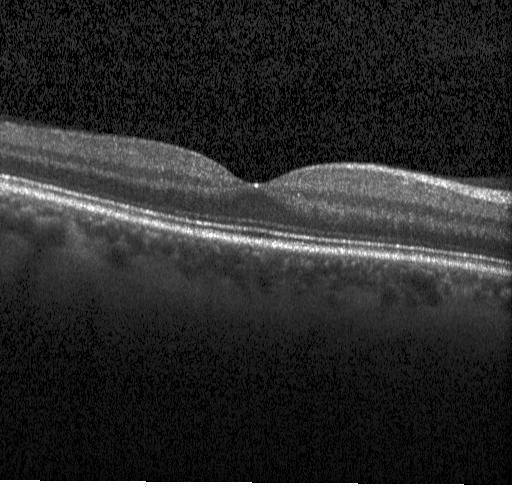 Macular OCT: no CNV, no DME, and no drusen.